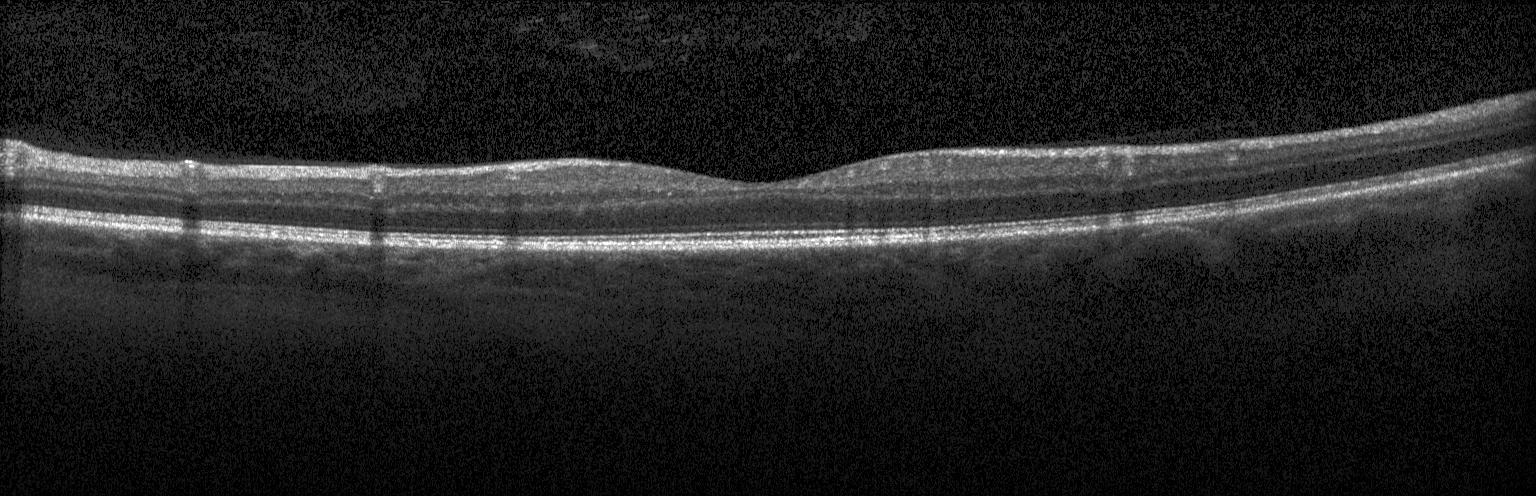

Impression: no choroidal neovascularization, no diabetic macular edema, and no drusen.